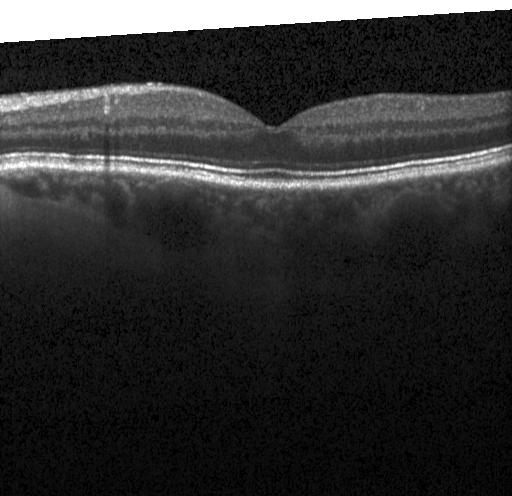
Macular scan; spectral-domain optical coherence tomography; OCT line scan; instrument: Heidelberg Spectralis
OCT finding: no evidence of choroidal neovascularization, diabetic macular edema, or drusen.